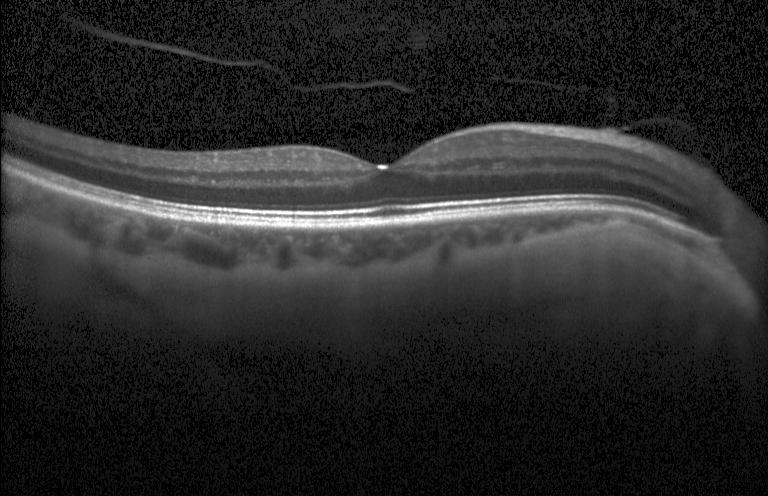
OCT line scan. Spectral-domain optical coherence tomography. Instrument: Heidelberg Spectralis. Centered on the fovea — Assessment: no choroidal neovascularization, diabetic macular edema, or drusen.